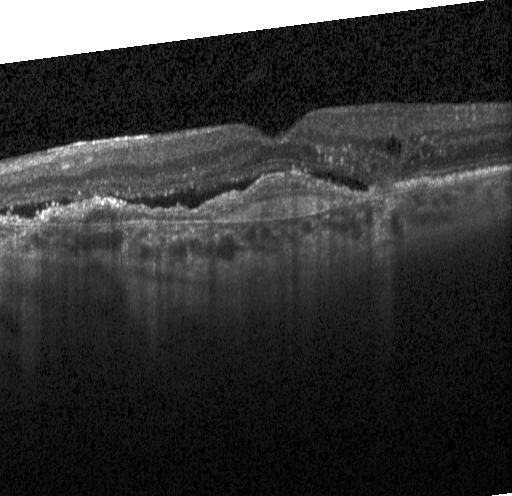

Acquired on a Heidelberg Spectralis. Optical coherence tomography B-scan
The scan shows a choroidal neovascular membrane.